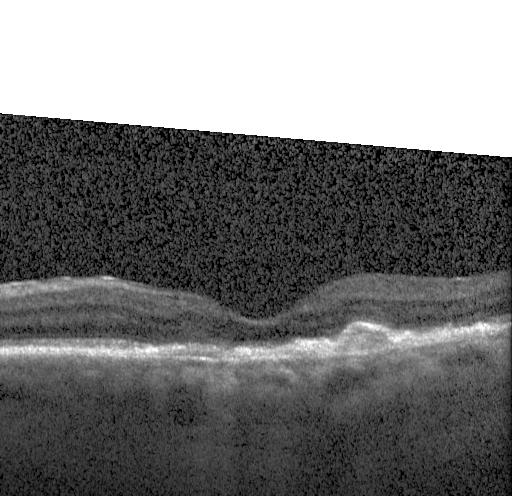

Acquired on a Heidelberg Spectralis; optical coherence tomography B-scan; spectral-domain OCT; fovea-centered — Impression: a choroidal neovascular membrane.